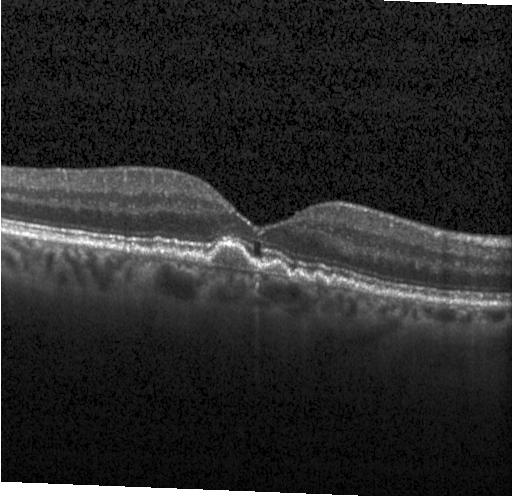
Through the macula · OCT line scan · spectral-domain OCT
This B-scan demonstrates drusen.